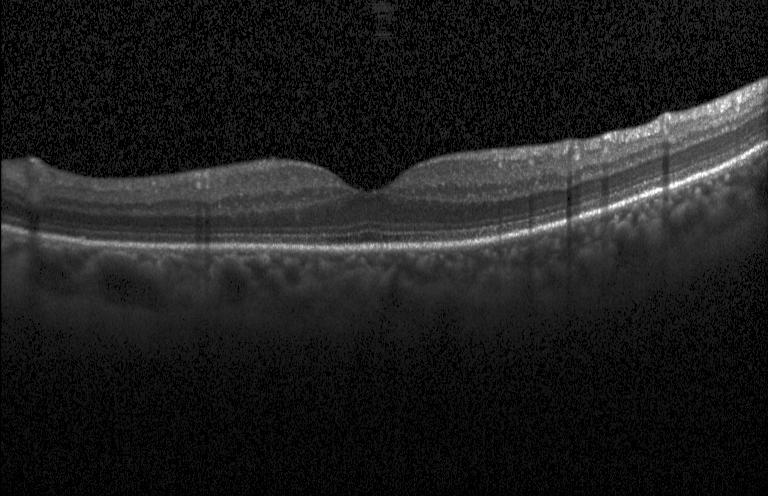
Dx: neither choroidal neovascularization, diabetic macular edema, nor drusen.